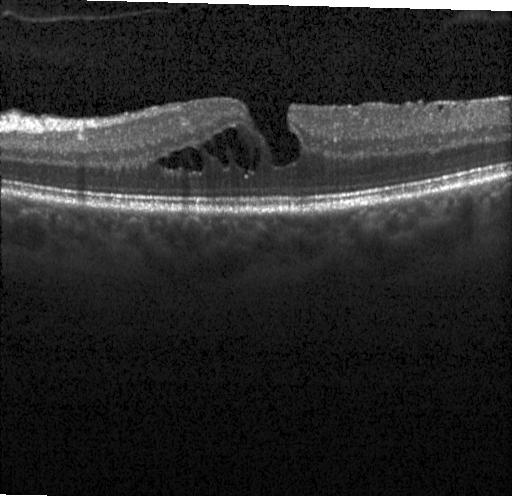

Optical coherence tomography B-scan
Impression: DME.